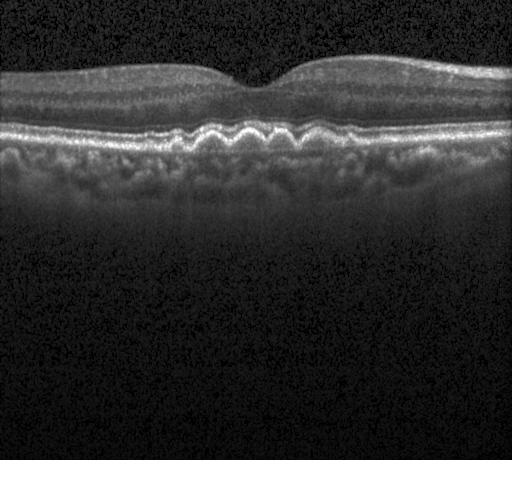

OCT B-scan. Spectral-domain OCT. Assessment: drusen.